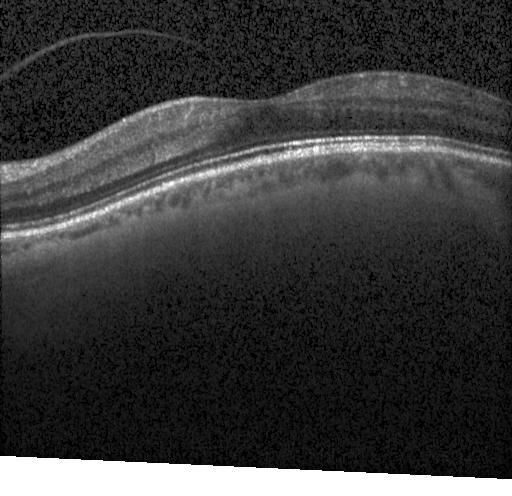
OCT finding: no evidence of choroidal neovascularization, diabetic macular edema, or drusen.